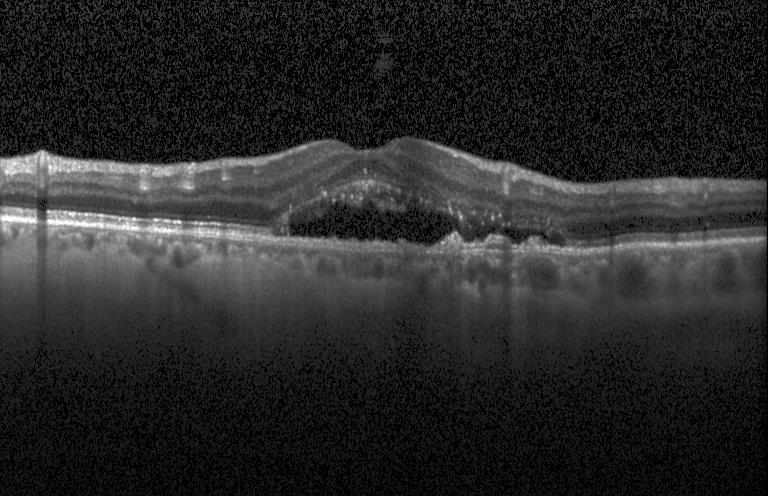

OCT finding: a choroidal neovascular membrane.